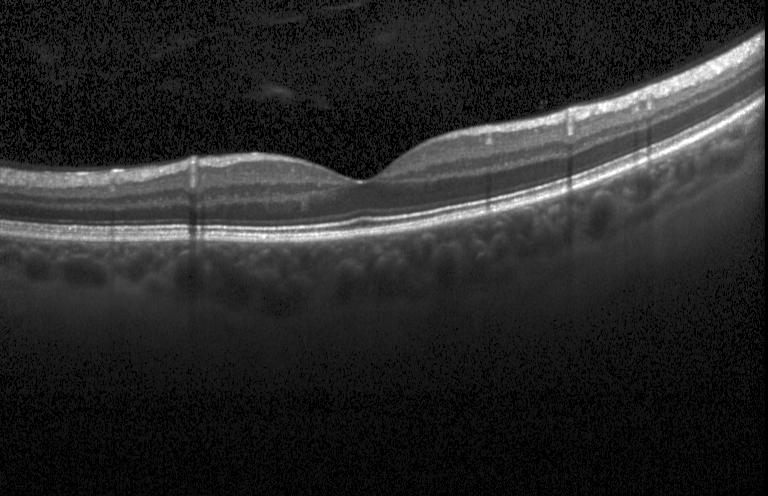
Acquired on a Heidelberg Spectralis; OCT line scan; horizontal scan through the fovea
Macular OCT: neither choroidal neovascularization, diabetic macular edema, nor drusen.